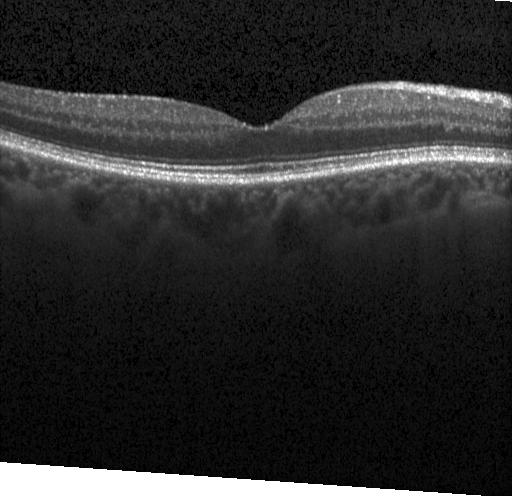
Heidelberg Spectralis OCT system · OCT line scan. This B-scan demonstrates no choroidal neovascularization, diabetic macular edema, or drusen.